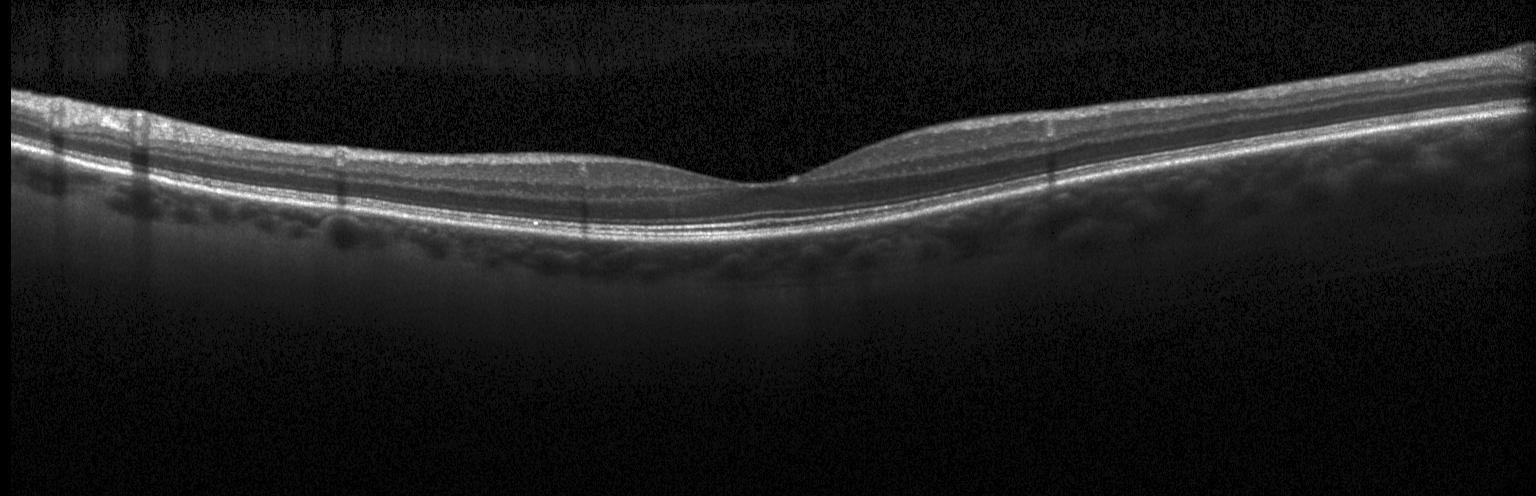 Optical coherence tomography scan — The scan shows no choroidal neovascularization, no diabetic macular edema, and no drusen.